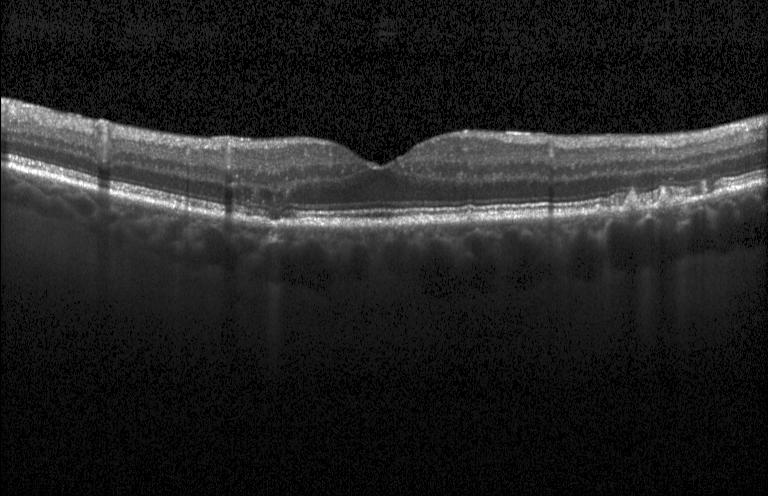
Spectral-domain optical coherence tomography; fovea-centered; retinal OCT cross-section
Assessment: sub-RPE drusenoid deposits.